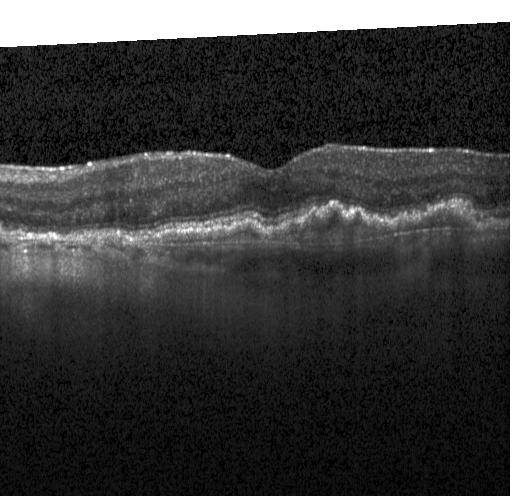
OCT B-scan. Acquired on a Heidelberg Spectralis. Centered on the fovea
The scan shows a choroidal neovascular membrane.